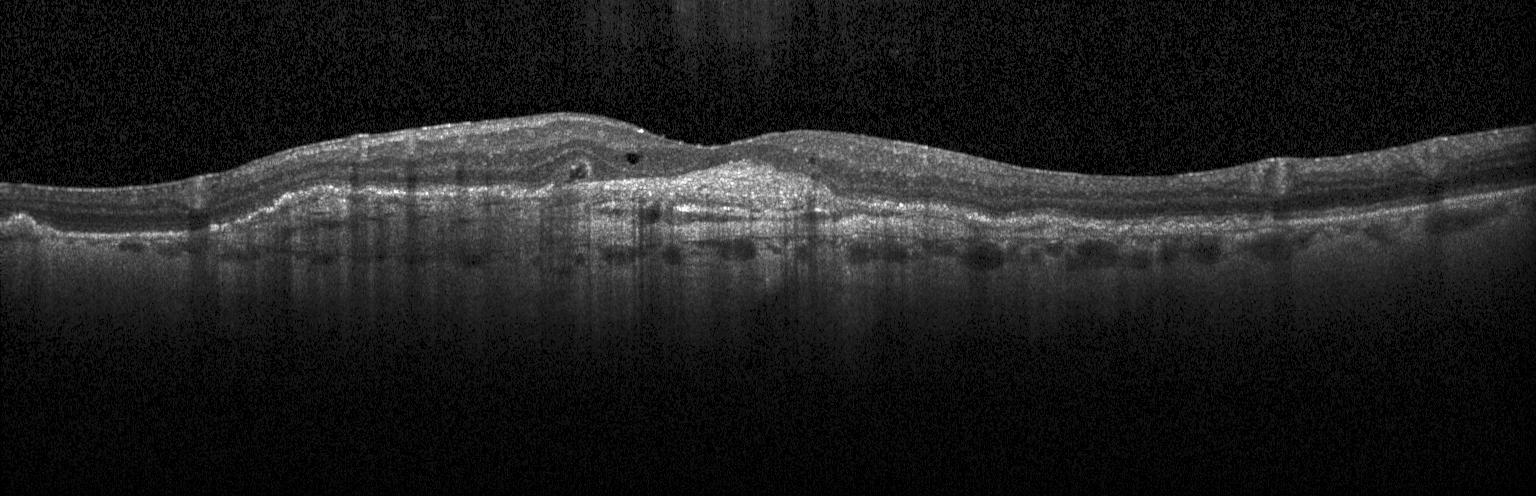 Diagnosis: a choroidal neovascular membrane.